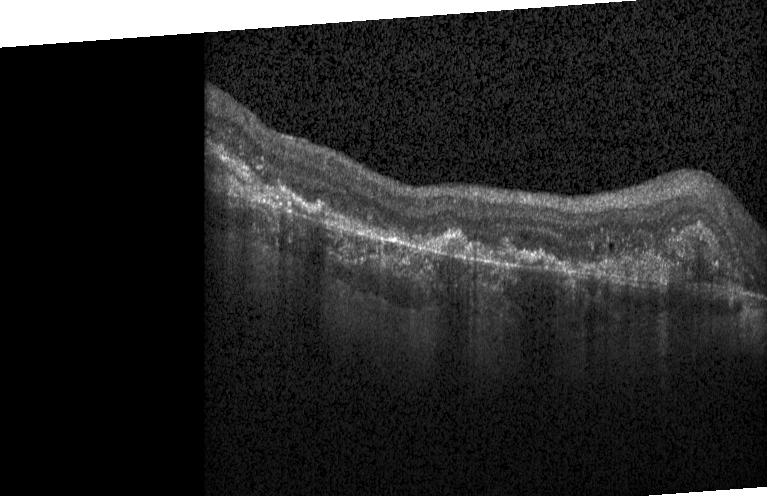

Instrument: Heidelberg Spectralis; OCT line scan; spectral-domain OCT — Impression: a choroidal neovascular membrane.